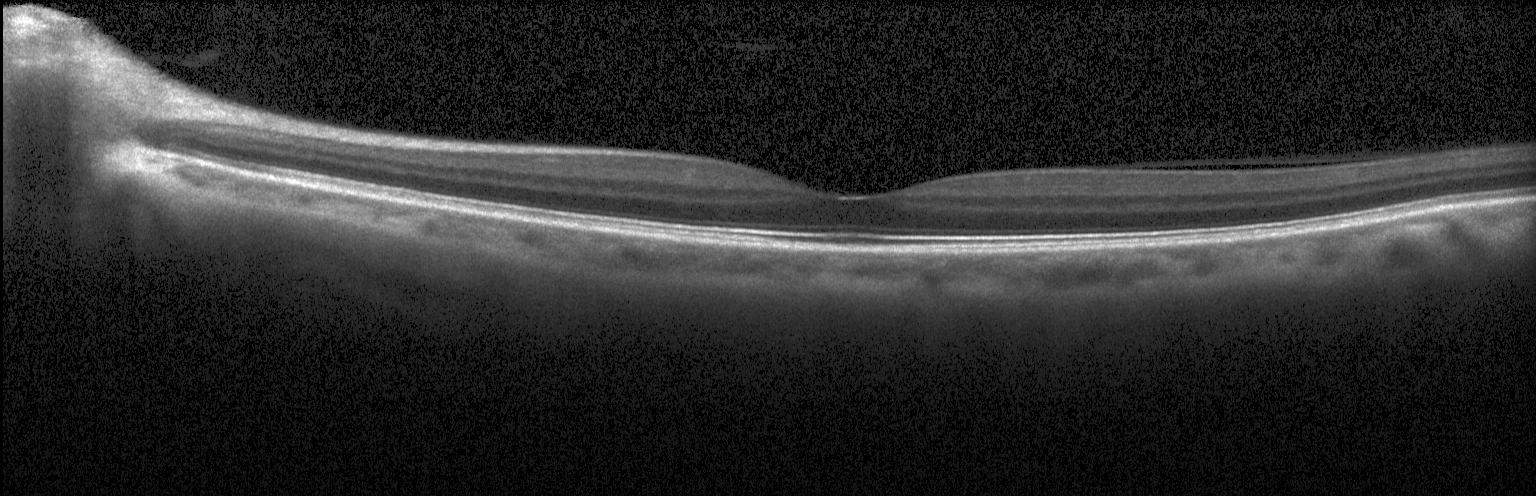
Impression: no evidence of CNV, DME, or drusen.